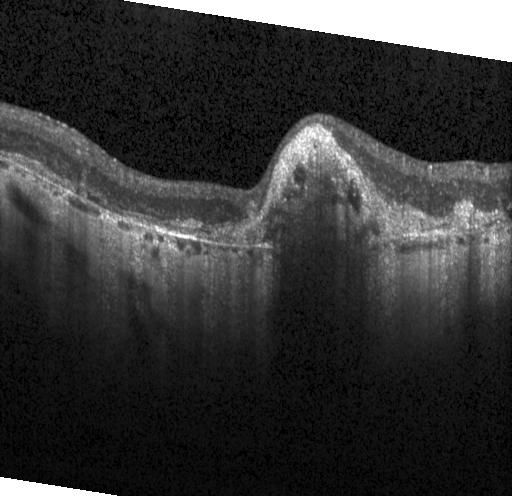 Finding: choroidal neovascularization (CNV).